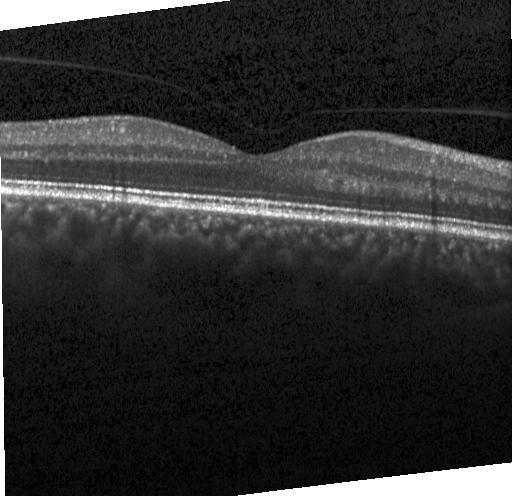

Retinal OCT cross-section; instrument: Heidelberg Spectralis; spectral-domain OCT; centered on the fovea
No CNV, DME, or drusen.